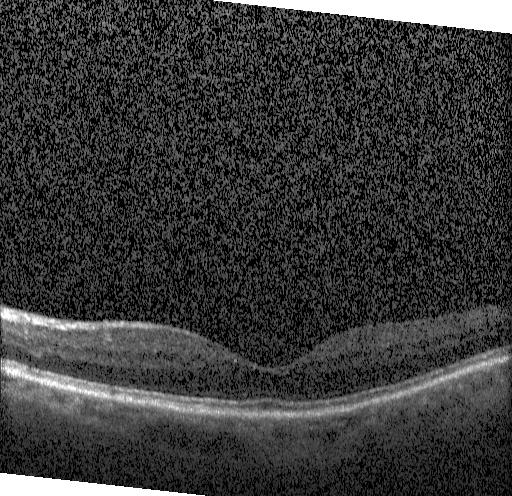
Finding: no evidence of CNV, DME, or drusen.